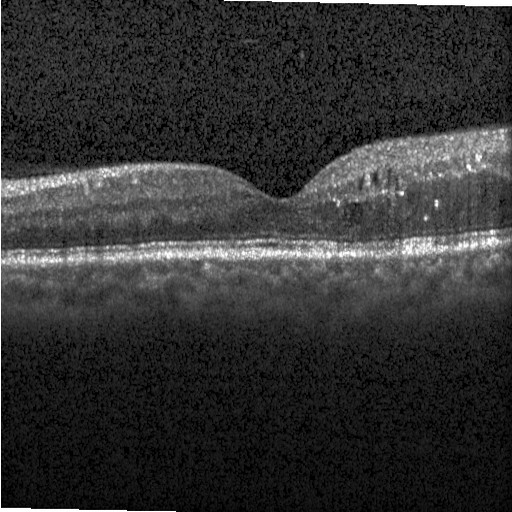 Optical coherence tomography B-scan · SD-OCT.
Assessment: DME.